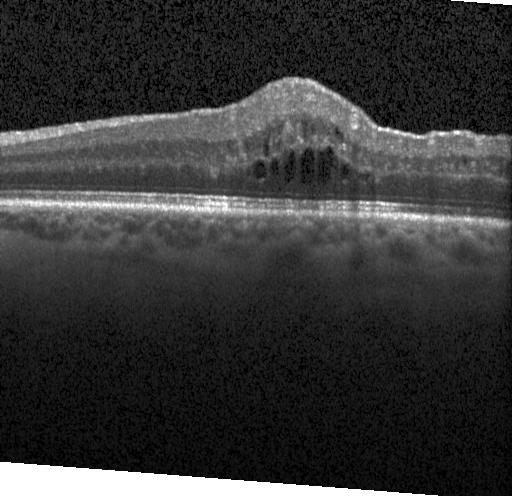 Impression: diabetic macular edema (DME).